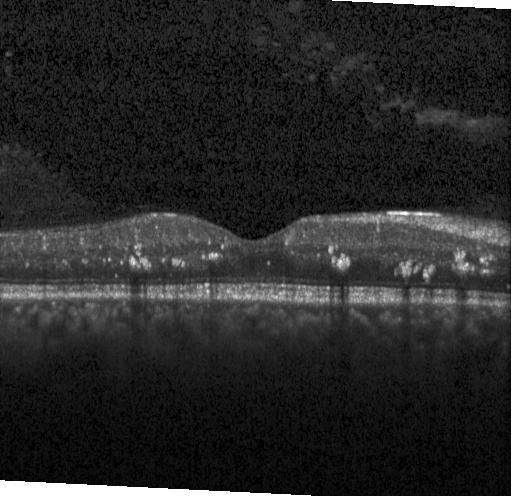

Diagnosis: DME.